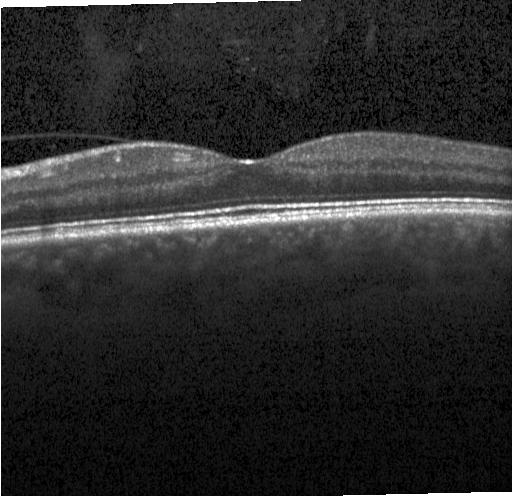 Horizontal scan through the fovea · Heidelberg Spectralis OCT system · spectral-domain optical coherence tomography · retinal OCT cross-section.
The scan shows neither choroidal neovascularization, diabetic macular edema, nor drusen.